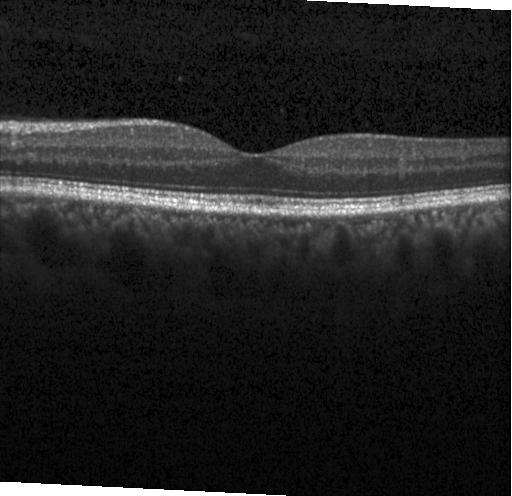

The scan shows no choroidal neovascularization, diabetic macular edema, or drusen.